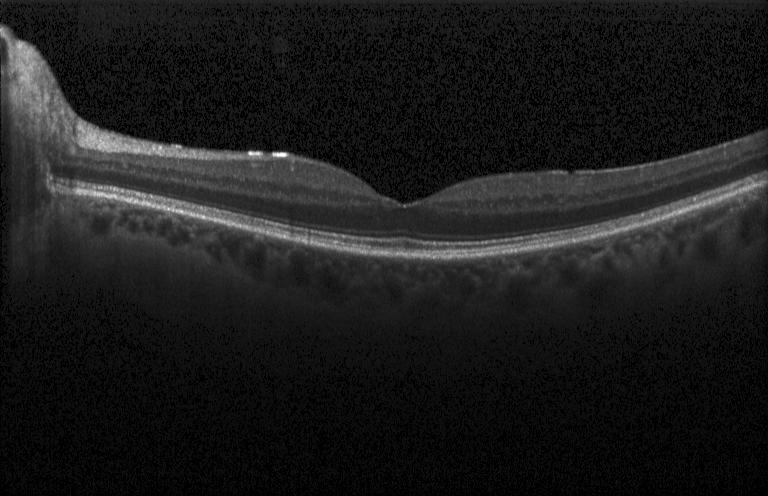

Optical coherence tomography B-scan; Heidelberg Spectralis. Macular OCT: no CNV, DME, or drusen.